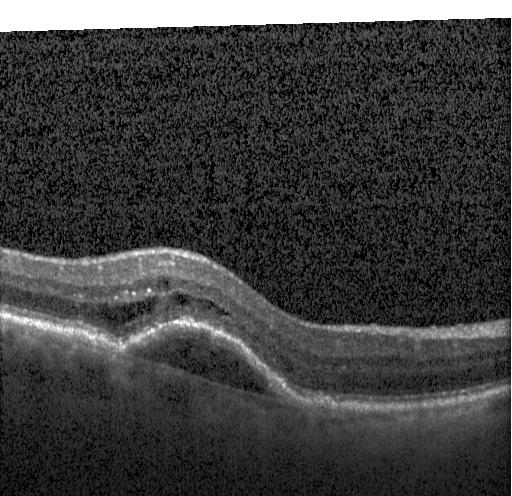
Retinal OCT cross-section showing a choroidal neovascular membrane.